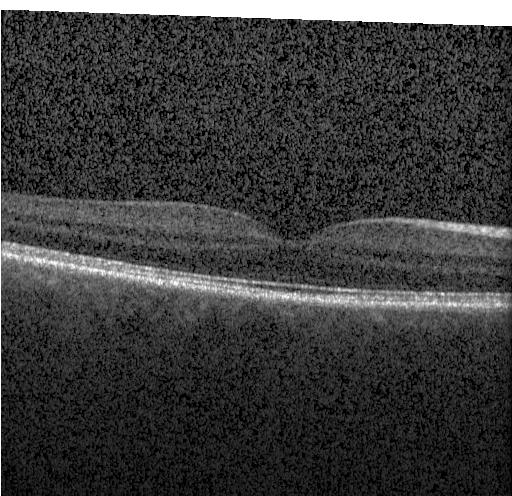 OCT B-scan. Macular OCT: no choroidal neovascularization, diabetic macular edema, or drusen.